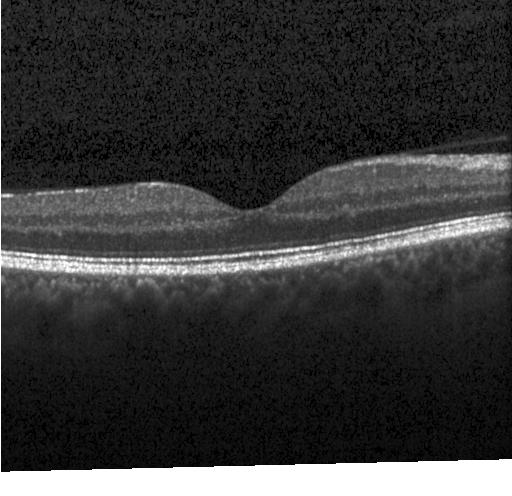 Optical coherence tomography scan. Spectral-domain OCT — Finding: neither CNV, DME, nor drusen.